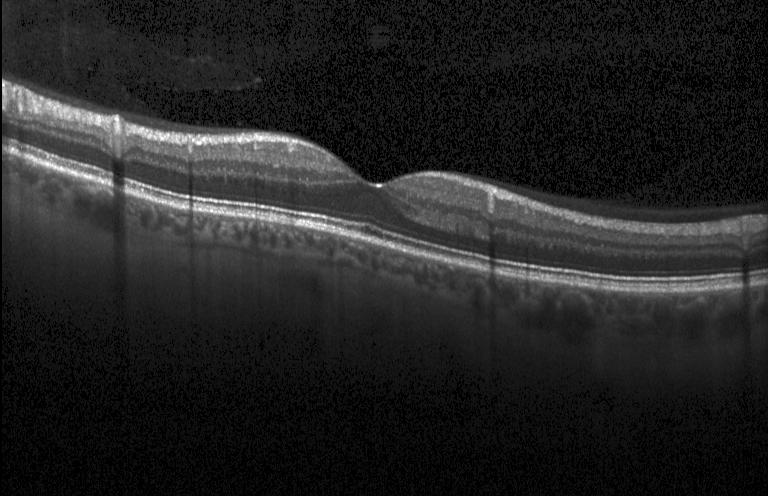

OCT line scan
This B-scan demonstrates no CNV, DME, or drusen.